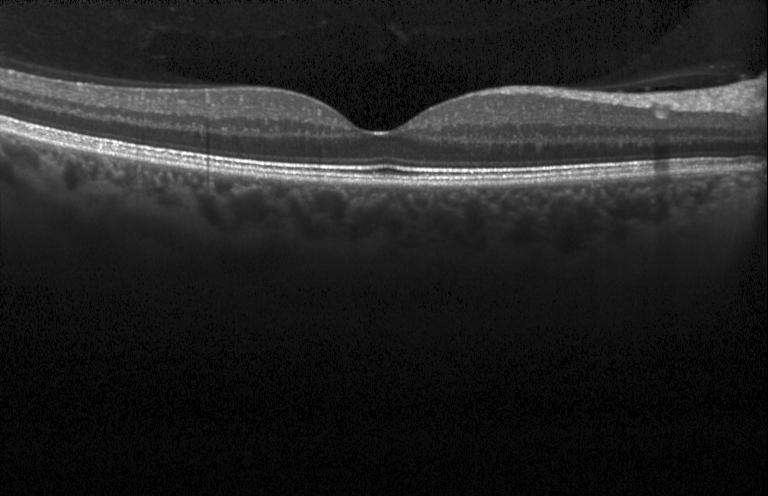 Optical coherence tomography scan; spectral-domain optical coherence tomography; horizontal scan through the fovea; Heidelberg Spectralis
Diagnosis: no choroidal neovascularization, no diabetic macular edema, and no drusen.